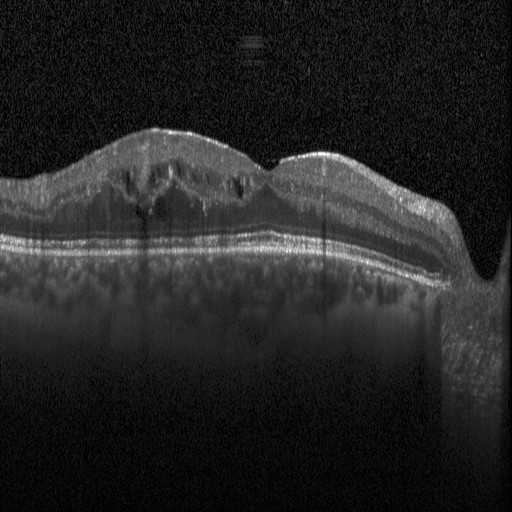
SD-OCT. Heidelberg Spectralis OCT system. OCT line scan — OCT finding: diabetic macular edema (DME).